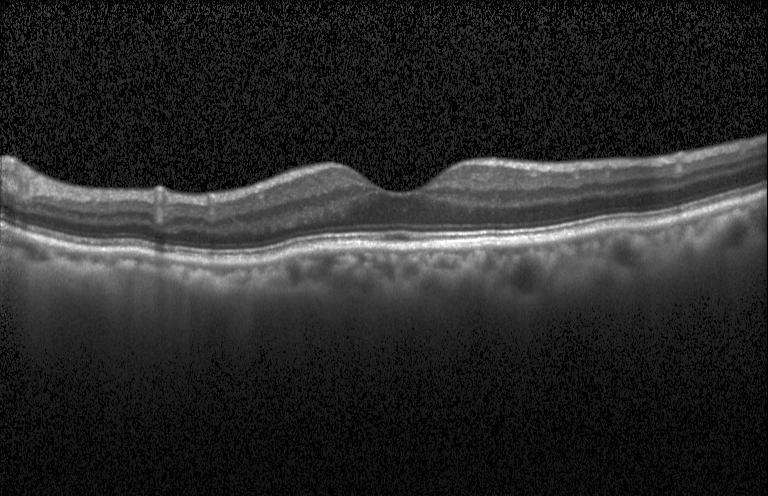

No choroidal neovascularization, no diabetic macular edema, and no drusen.